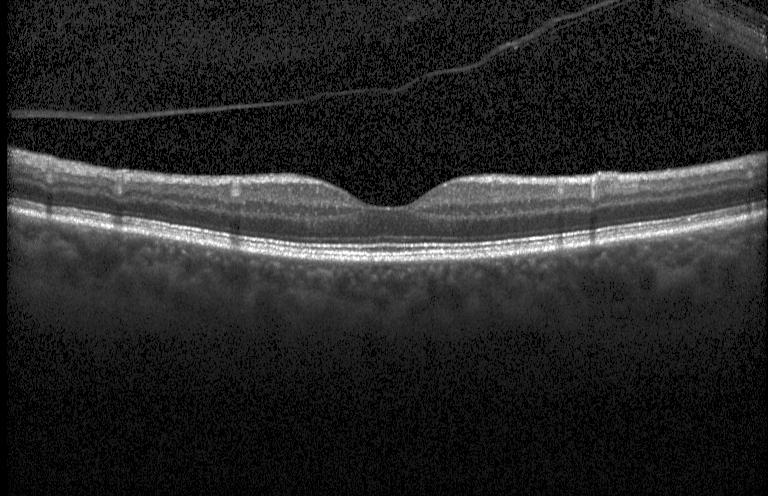

Fovea-centered, optical coherence tomography B-scan
Diagnosis: neither CNV, DME, nor drusen.